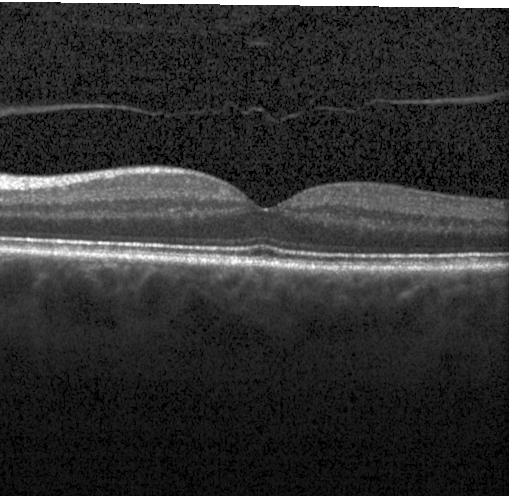
Optical coherence tomography scan · Heidelberg Spectralis OCT system.
The scan shows no evidence of choroidal neovascularization, diabetic macular edema, or drusen.